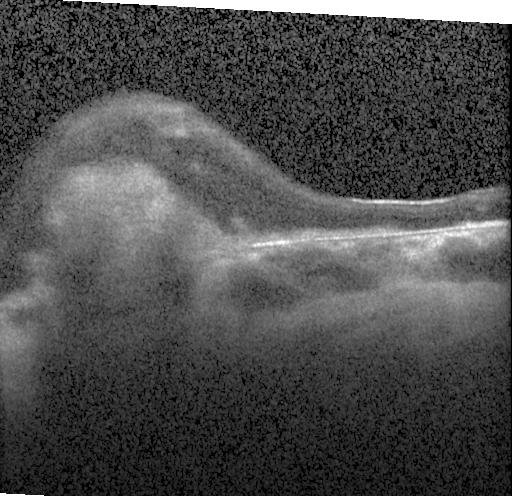
Spectral-domain optical coherence tomography. Optical coherence tomography B-scan. Fovea-centered.
Diagnosis: a choroidal neovascular membrane.